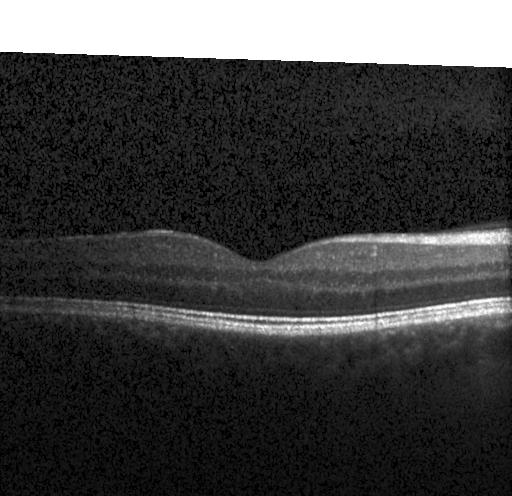 Fovea-centered; OCT line scan.
Diagnosis: no evidence of CNV, DME, or drusen.